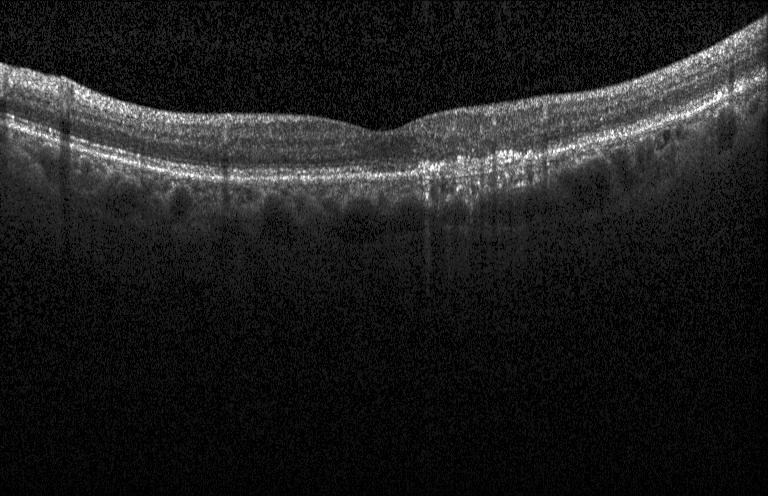
Heidelberg Spectralis OCT system; spectral-domain OCT; through the macula; OCT B-scan.
Macular OCT: a choroidal neovascular membrane.